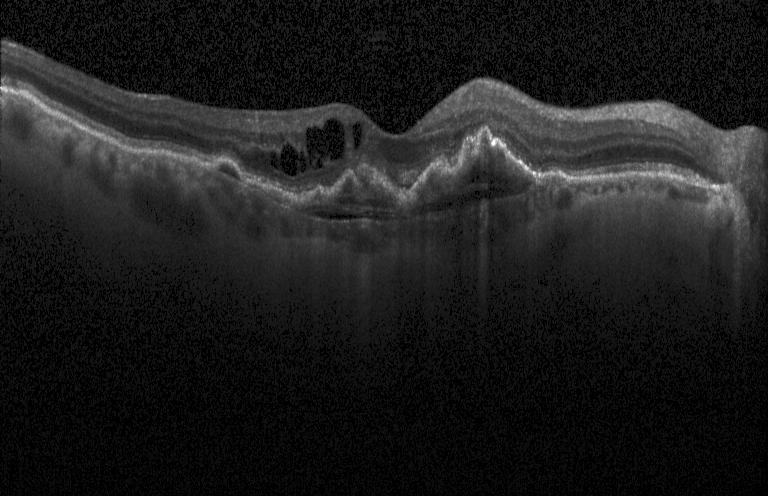

Retinal OCT B-scan. Heidelberg Spectralis — This B-scan demonstrates a choroidal neovascular membrane.